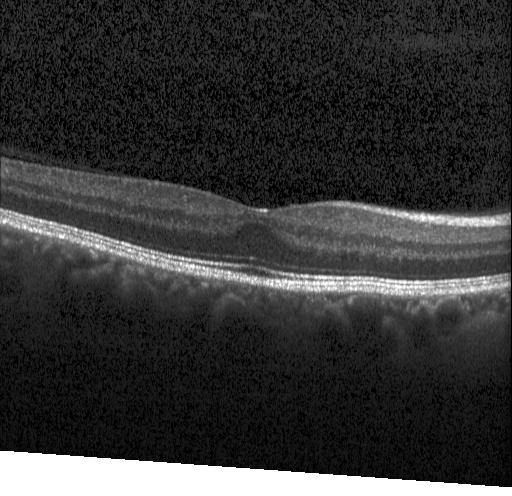 Fovea-centered, acquired on a Heidelberg Spectralis, OCT line scan
The scan shows neither CNV, DME, nor drusen.